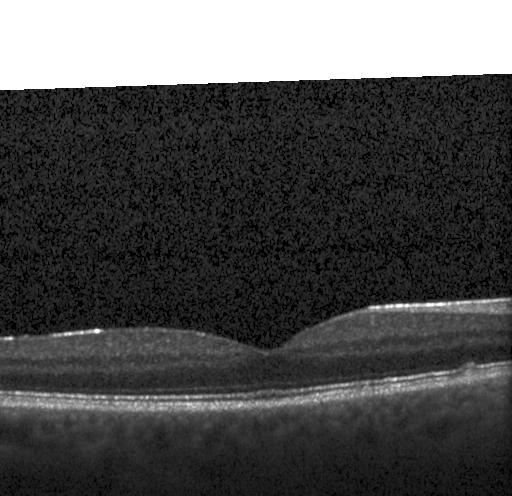
Horizontal scan through the fovea; OCT line scan; spectral-domain optical coherence tomography. OCT finding: drusen.